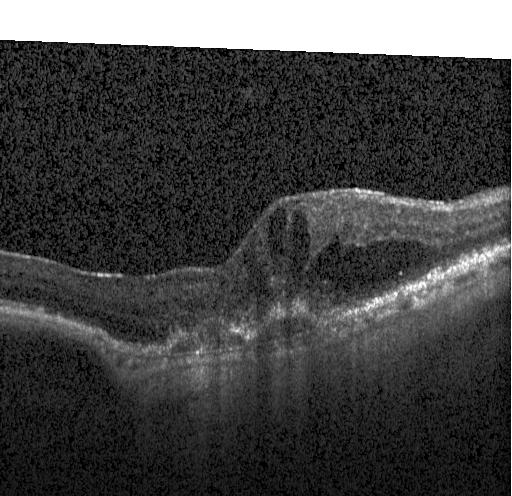
Macular scan. Spectral-domain optical coherence tomography. OCT B-scan. Heidelberg Spectralis OCT system — Diagnosis: a choroidal neovascular membrane.